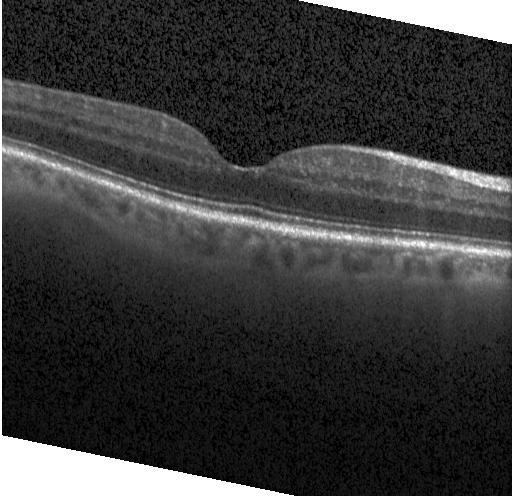
Dx: neither choroidal neovascularization, diabetic macular edema, nor drusen.